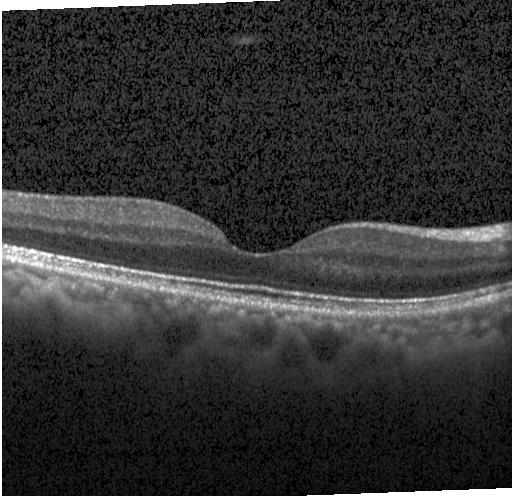 Finding: no choroidal neovascularization, no diabetic macular edema, and no drusen.